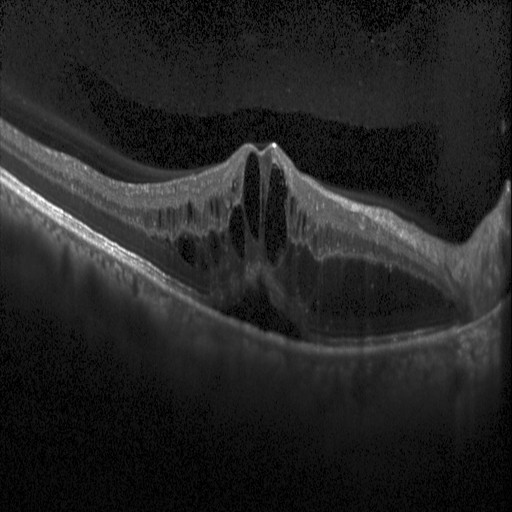 Acquired on a Heidelberg Spectralis, horizontal scan through the fovea, optical coherence tomography scan — DME.